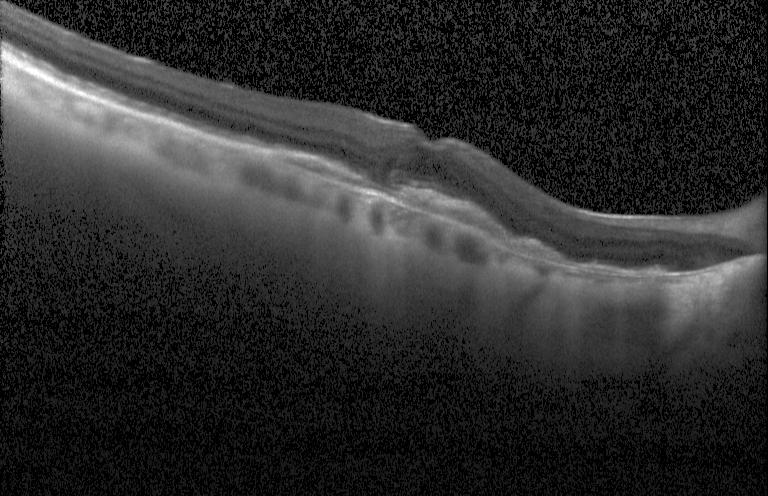

Optical coherence tomography B-scan · instrument: Heidelberg Spectralis.
Impression: a choroidal neovascular membrane.